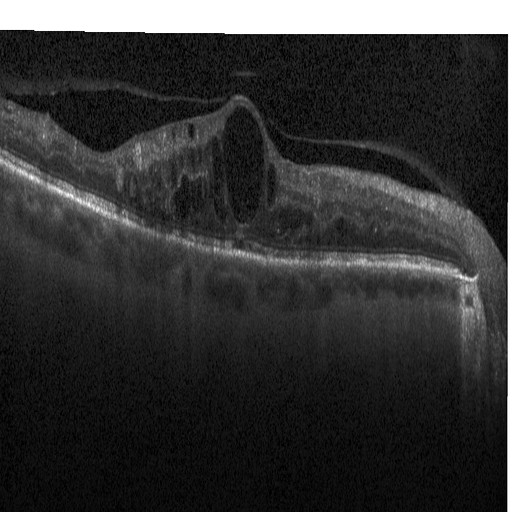 OCT B-scan
The scan shows diabetic macular edema (DME).